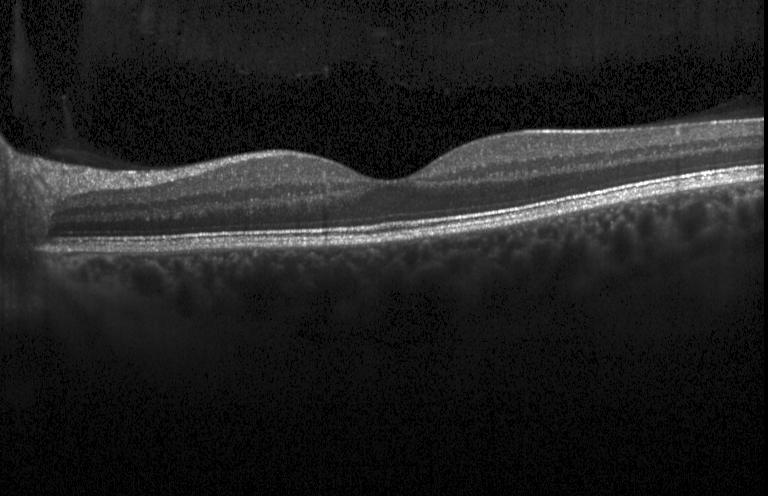
OCT B-scan. Neither choroidal neovascularization, diabetic macular edema, nor drusen.